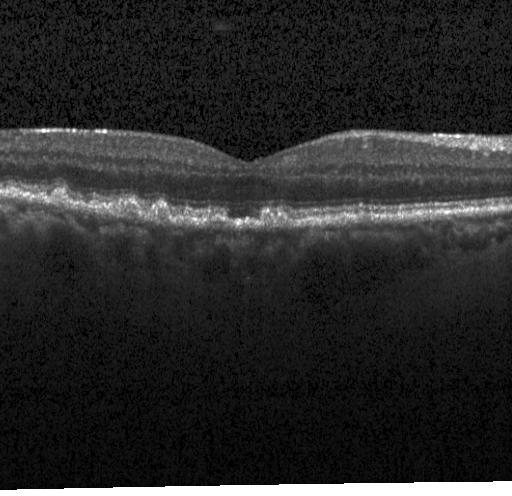 Finding: sub-RPE drusenoid deposits.